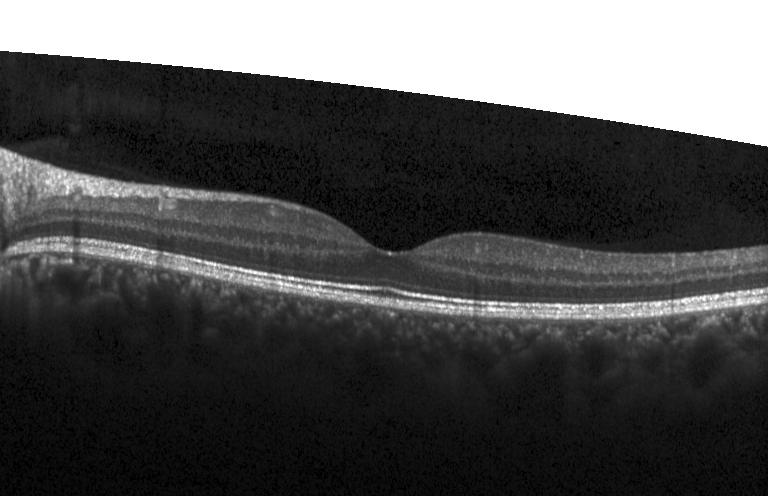
Fovea-centered · retinal OCT cross-section — The scan shows no evidence of choroidal neovascularization, diabetic macular edema, or drusen.